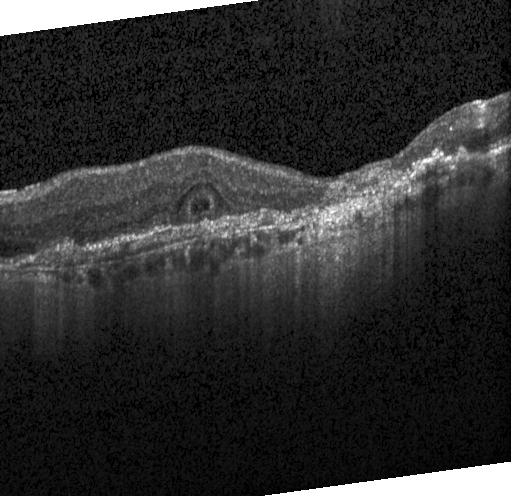 Heidelberg Spectralis OCT system, through the macula, optical coherence tomography B-scan — Diagnosis: choroidal neovascularization (CNV).